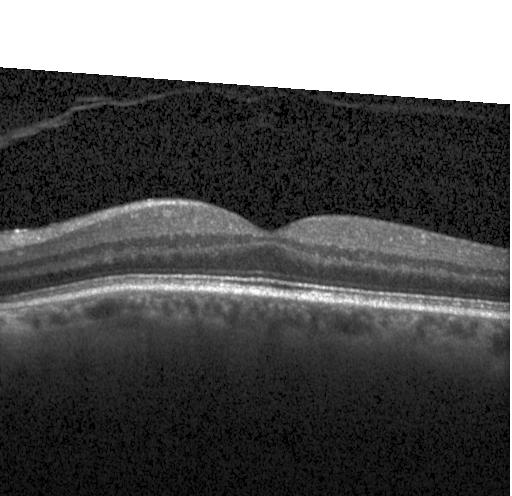 Retinal OCT cross-section; Heidelberg Spectralis OCT system; SD-OCT; fovea-centered. OCT finding: no CNV, DME, or drusen.